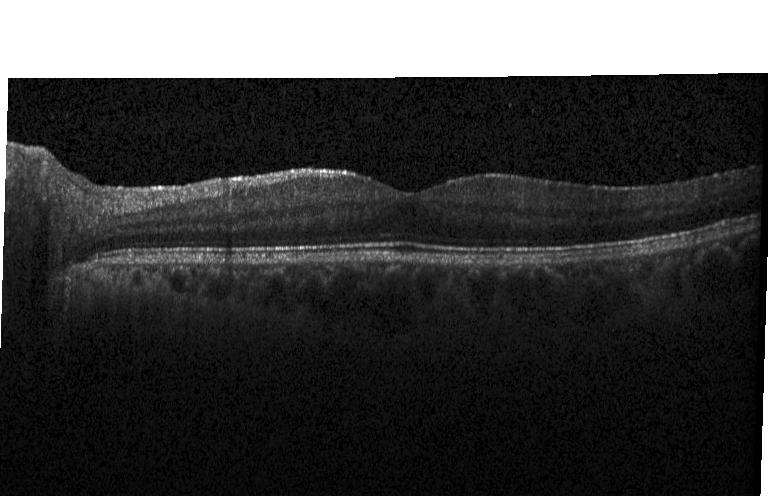
Retinal OCT cross-section showing no evidence of choroidal neovascularization, diabetic macular edema, or drusen.